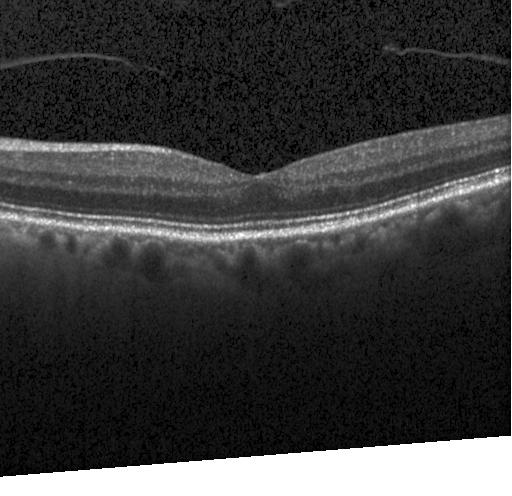

Impression: no CNV, DME, or drusen.